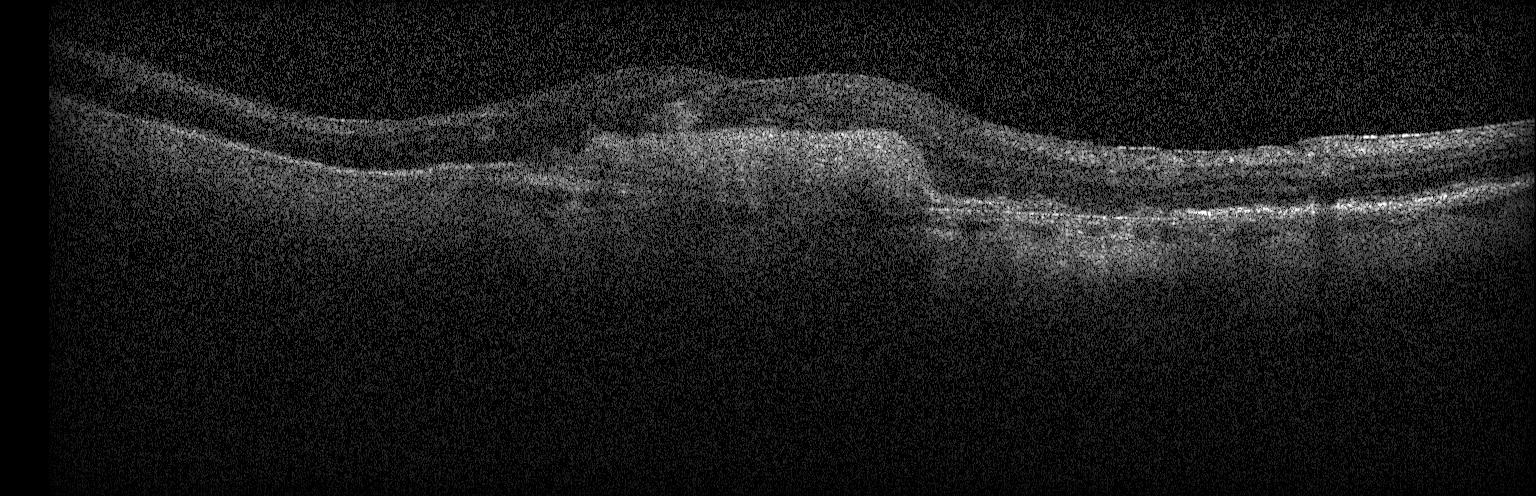 SD-OCT; retinal OCT B-scan; fovea-centered; acquired on a Heidelberg Spectralis. Choroidal neovascularization.